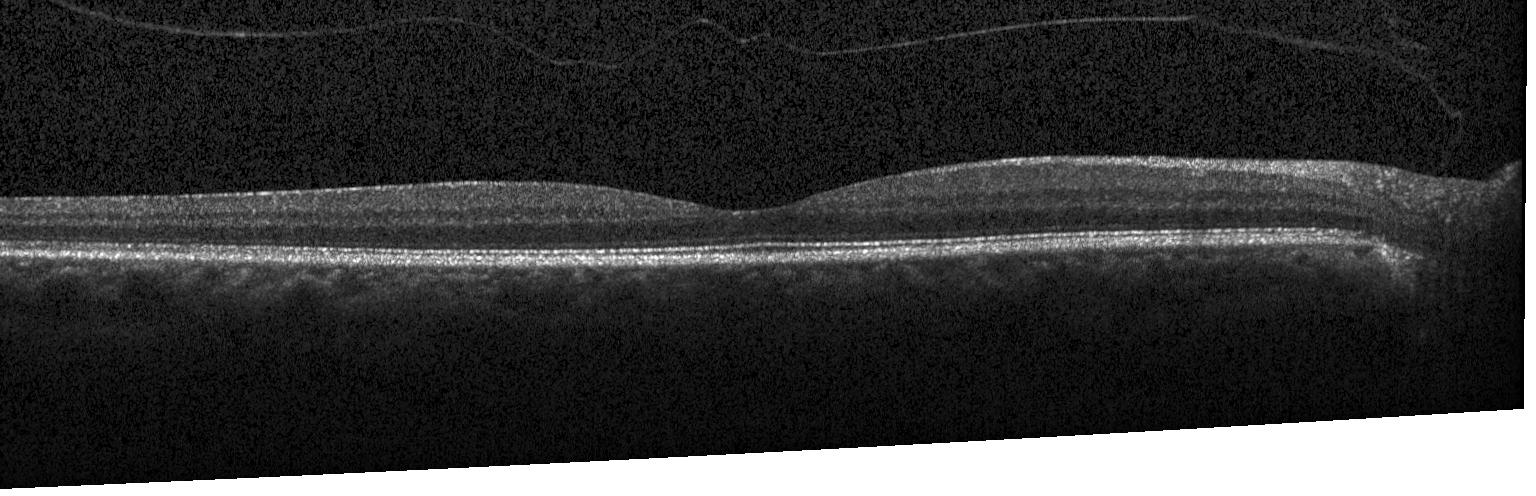
Retinal OCT B-scan. Spectral-domain optical coherence tomography. Instrument: Heidelberg Spectralis. Horizontal scan through the fovea
Macular OCT: no evidence of CNV, DME, or drusen.